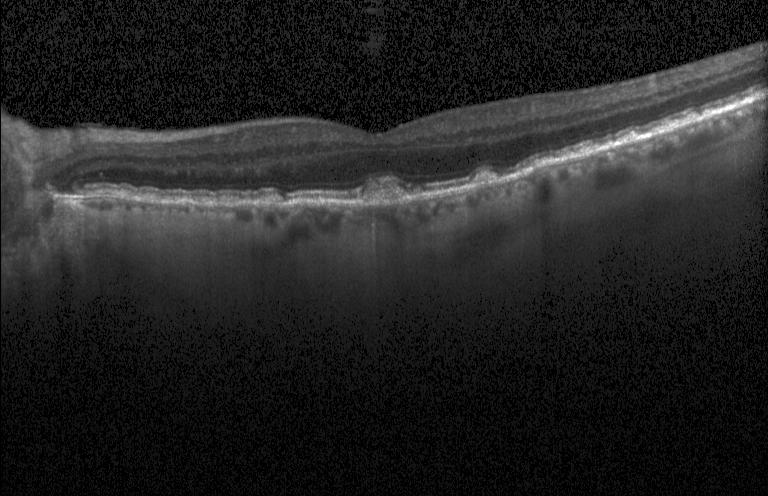
Finding: sub-RPE drusenoid deposits.